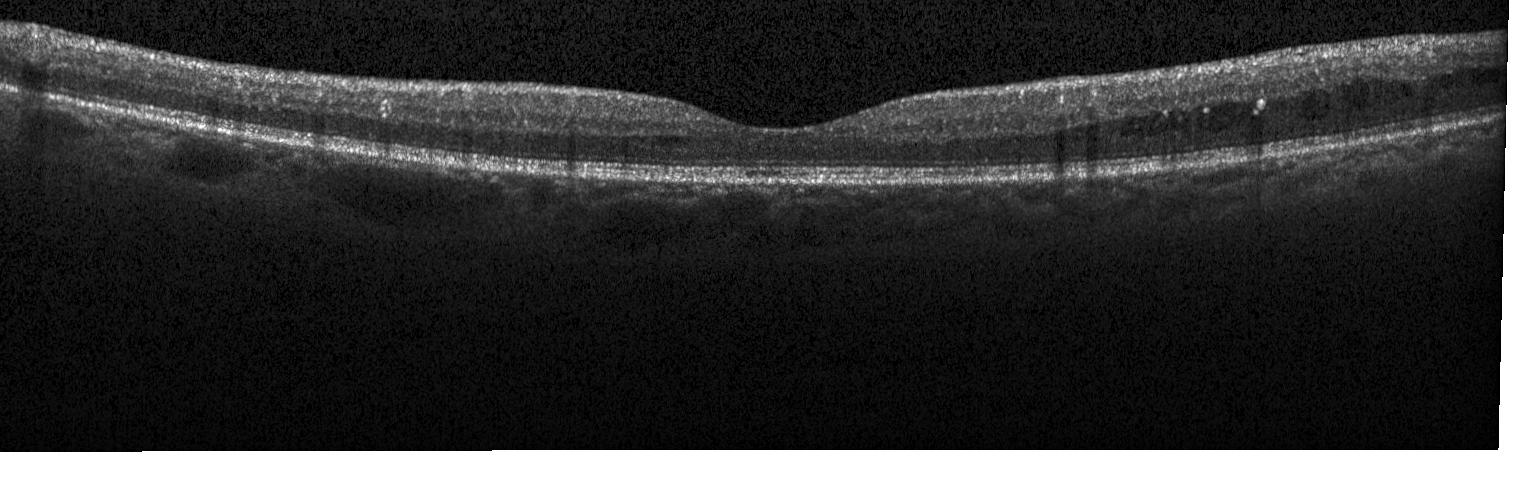
Retinal OCT cross-section showing neither choroidal neovascularization, diabetic macular edema, nor drusen.